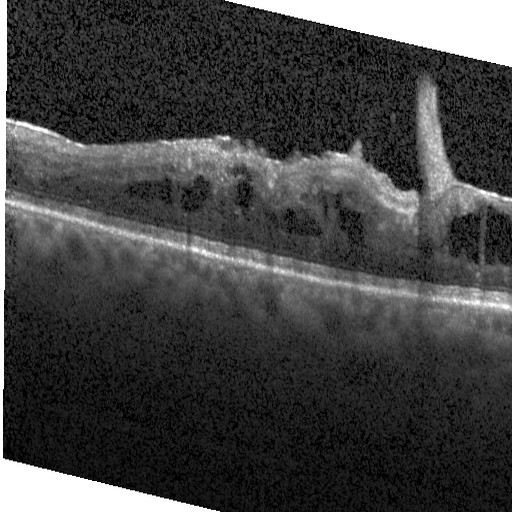

Acquired on a Heidelberg Spectralis; optical coherence tomography scan. Assessment: DME.